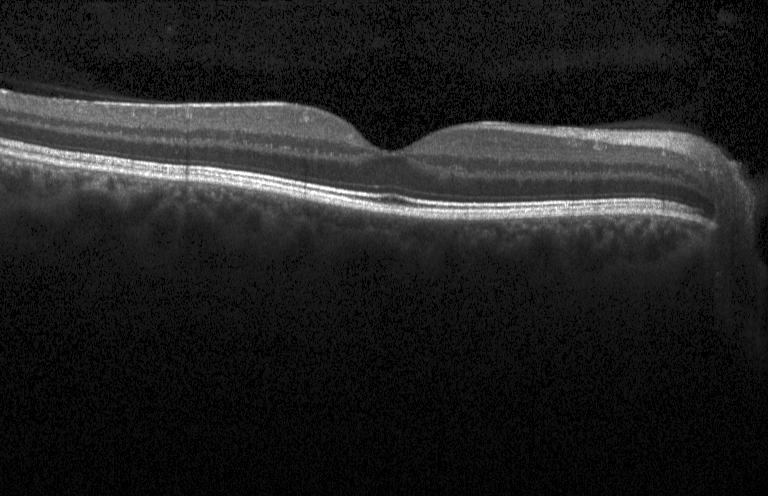
Diagnosis: no choroidal neovascularization, no diabetic macular edema, and no drusen.